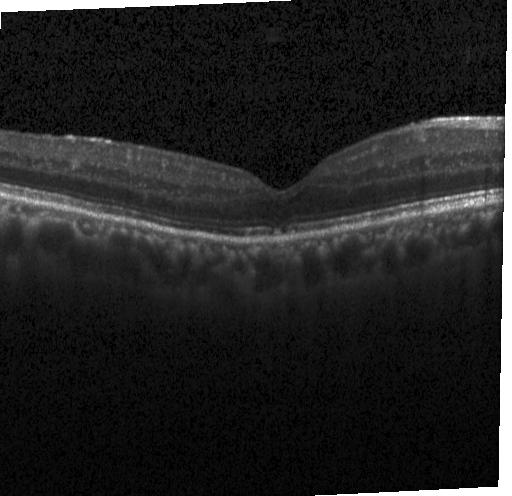
Optical coherence tomography B-scan. Heidelberg Spectralis.
The scan shows no choroidal neovascularization, diabetic macular edema, or drusen.